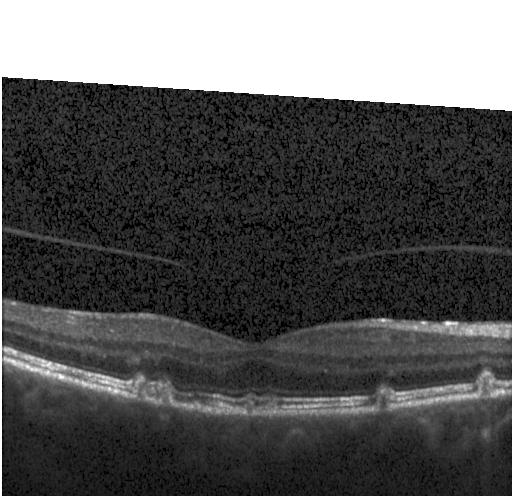

Retinal OCT cross-section showing sub-RPE drusenoid deposits.